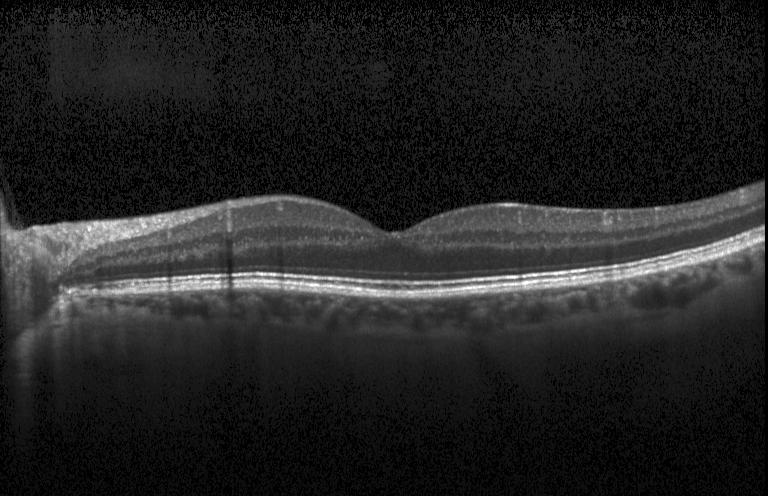

Instrument: Heidelberg Spectralis · optical coherence tomography scan
Diagnosis: neither choroidal neovascularization, diabetic macular edema, nor drusen.